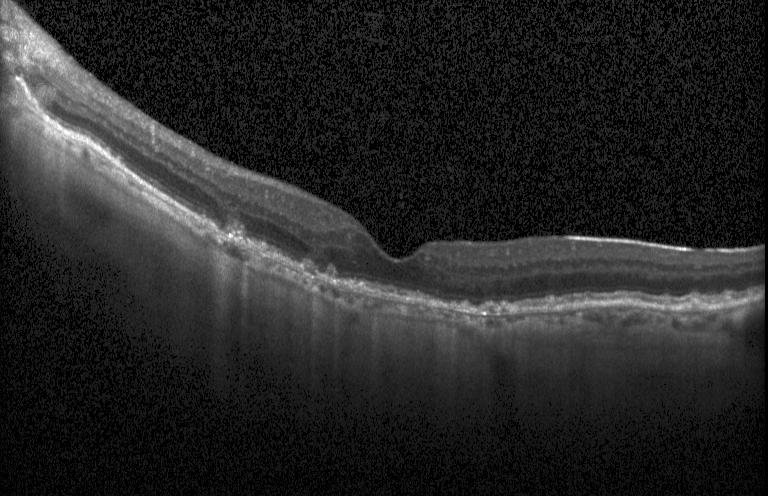

OCT B-scan.
This B-scan demonstrates choroidal neovascularization (CNV).